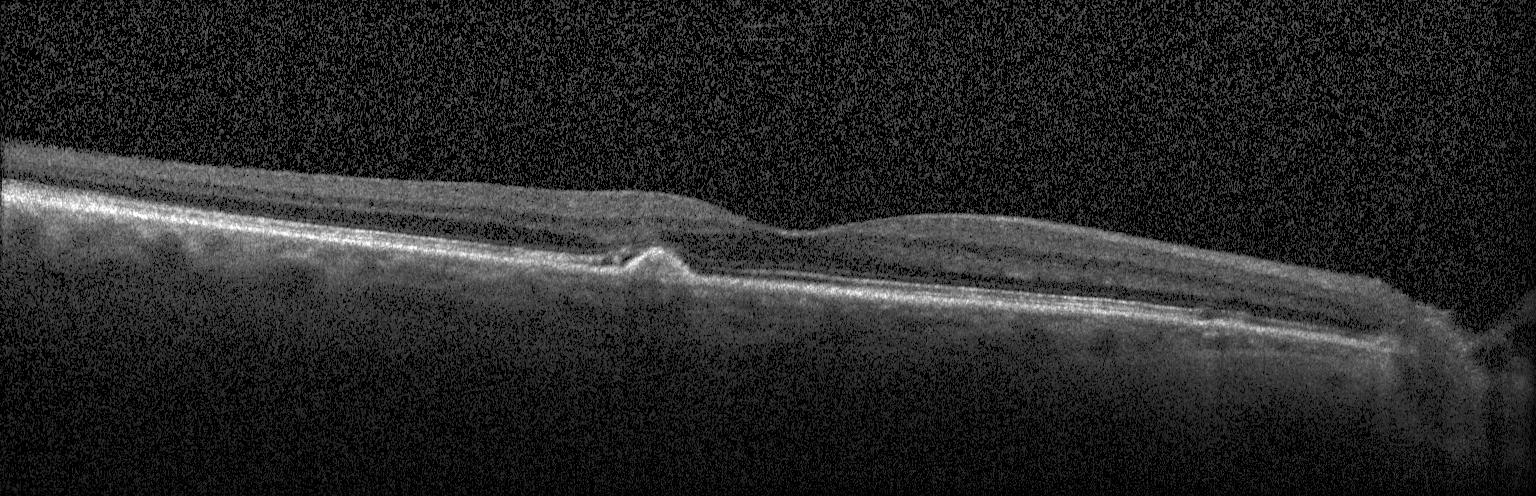
Macular OCT demonstrating CNV.